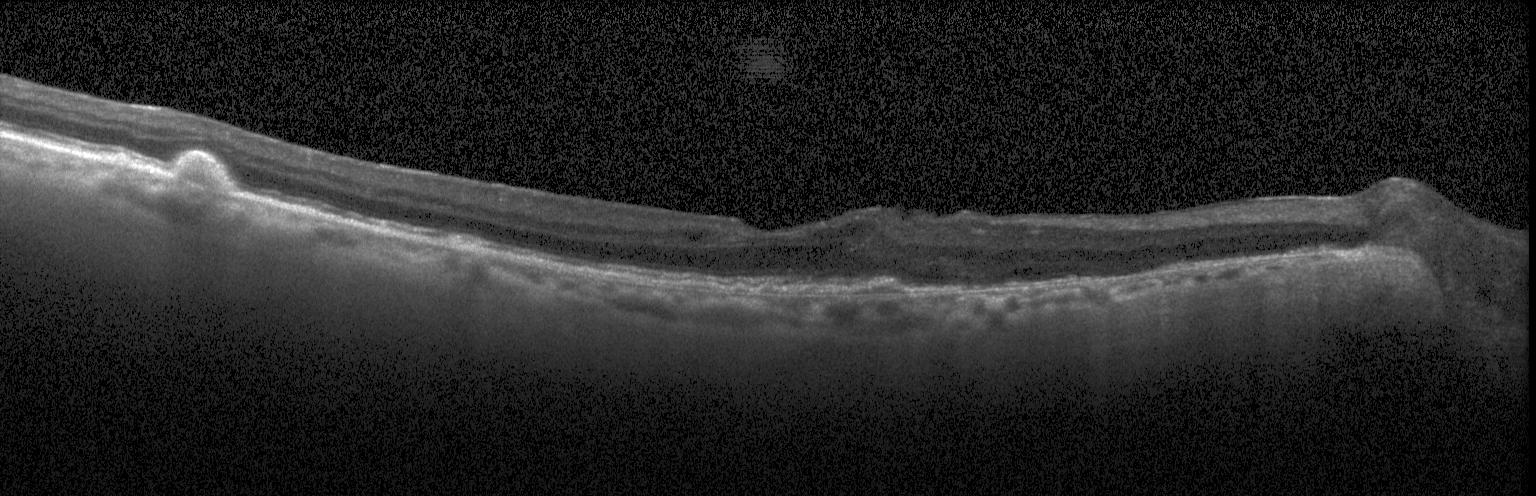 Horizontal scan through the fovea. Heidelberg Spectralis OCT system. Optical coherence tomography scan.
Macular OCT: a choroidal neovascular membrane.